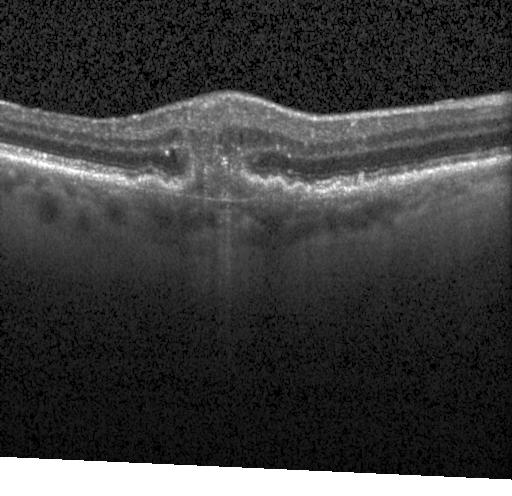

Macular OCT: choroidal neovascularization.